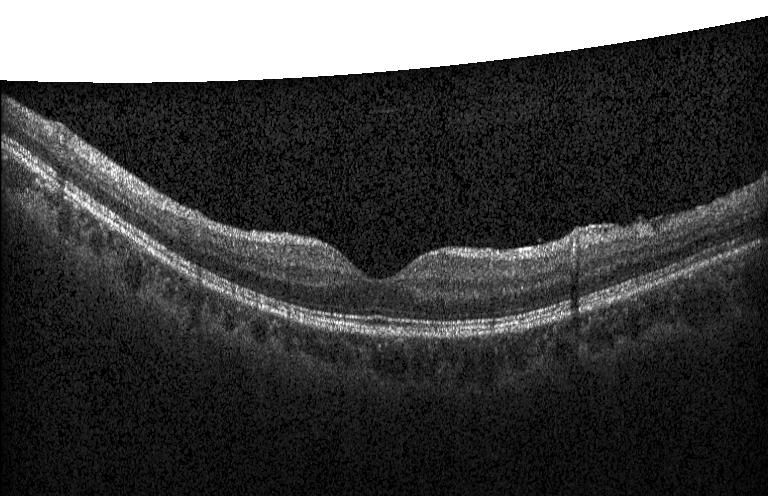

OCT B-scan showing no choroidal neovascularization, no diabetic macular edema, and no drusen.